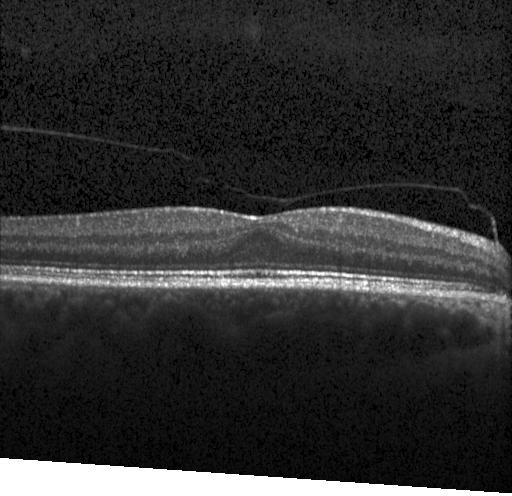
Through the macula · optical coherence tomography B-scan. Macular OCT: no choroidal neovascularization, no diabetic macular edema, and no drusen.